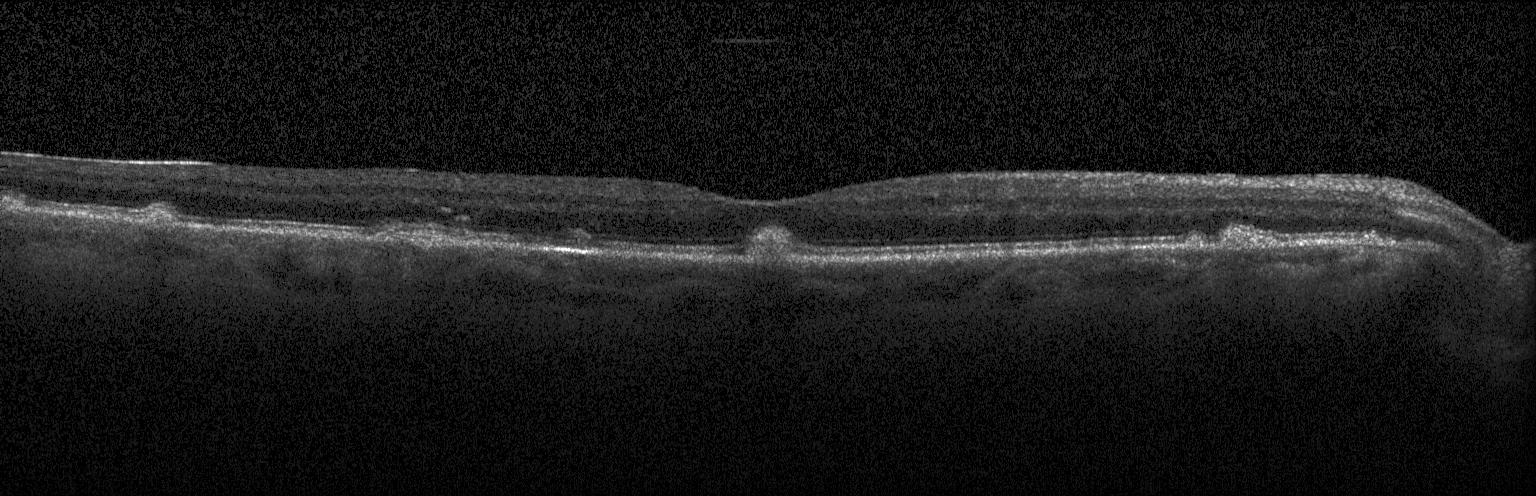

Instrument: Heidelberg Spectralis · through the macula · OCT B-scan.
Finding: multiple drusen.